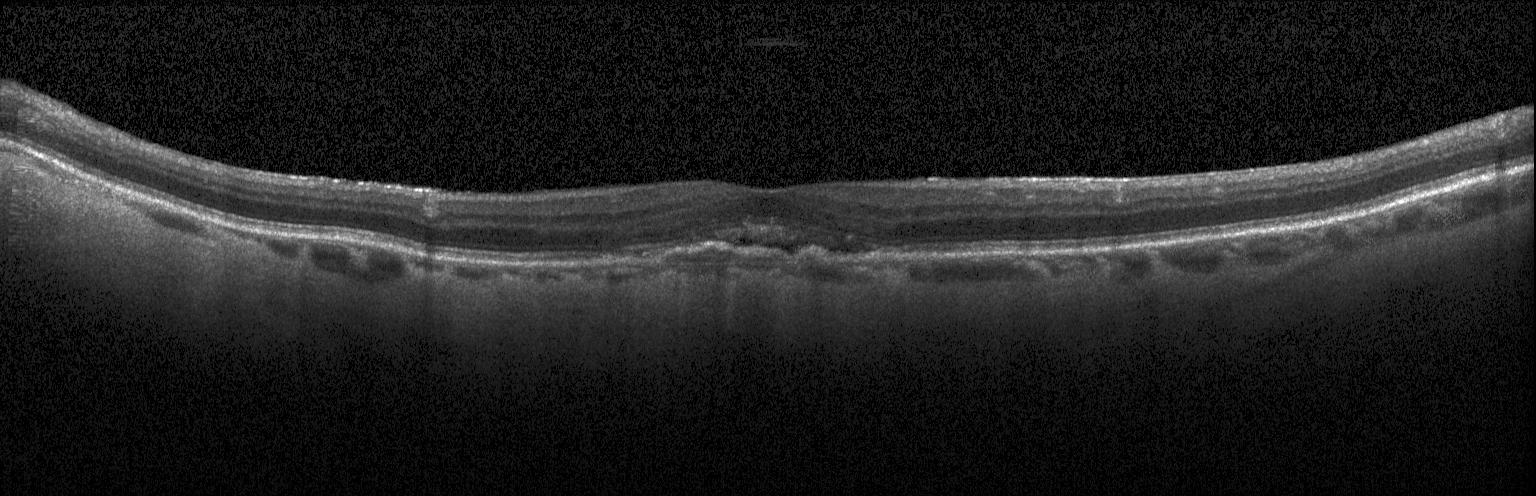

Retinal OCT cross-section · fovea-centered · SD-OCT
Dx: a choroidal neovascular membrane.